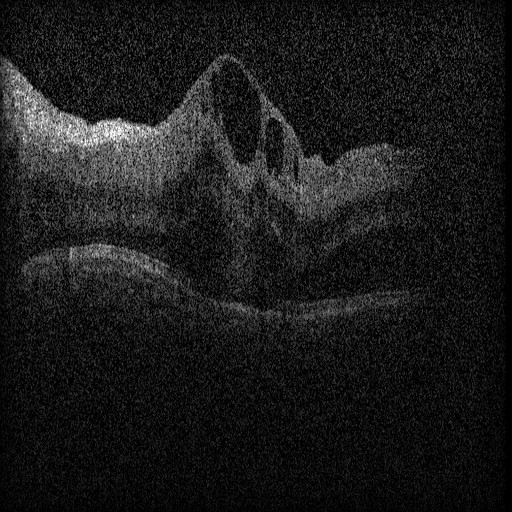
Impression: diabetic macular edema (DME).